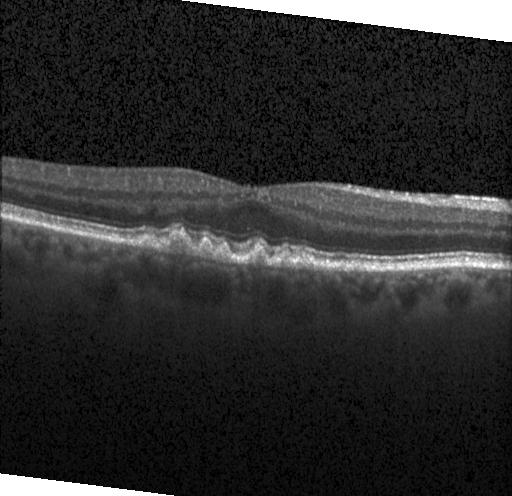 Multiple drusen.